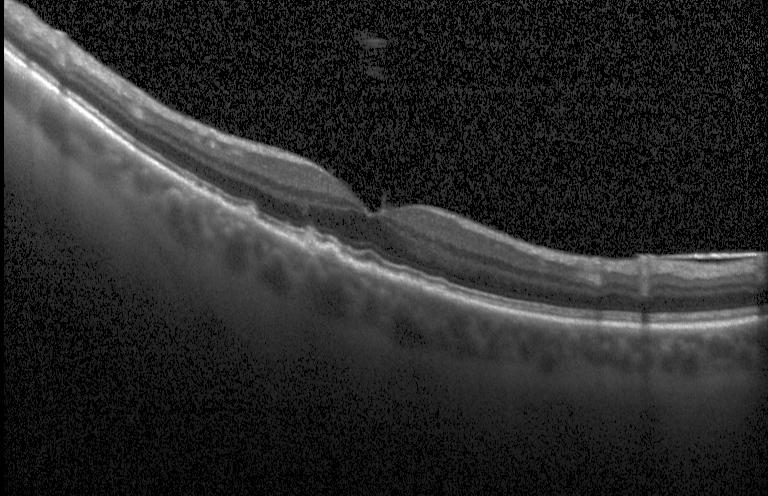
Optical coherence tomography scan, spectral-domain optical coherence tomography, Heidelberg Spectralis OCT system, horizontal scan through the fovea.
Impression: multiple drusen.